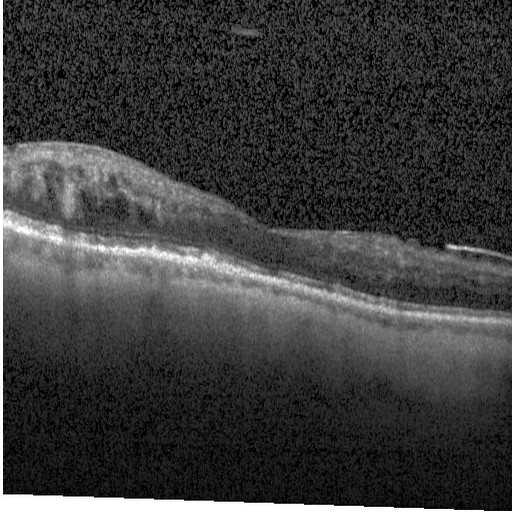

Retinal OCT cross-section · spectral-domain OCT · macular scan · instrument: Heidelberg Spectralis
Finding: diabetic macular edema.